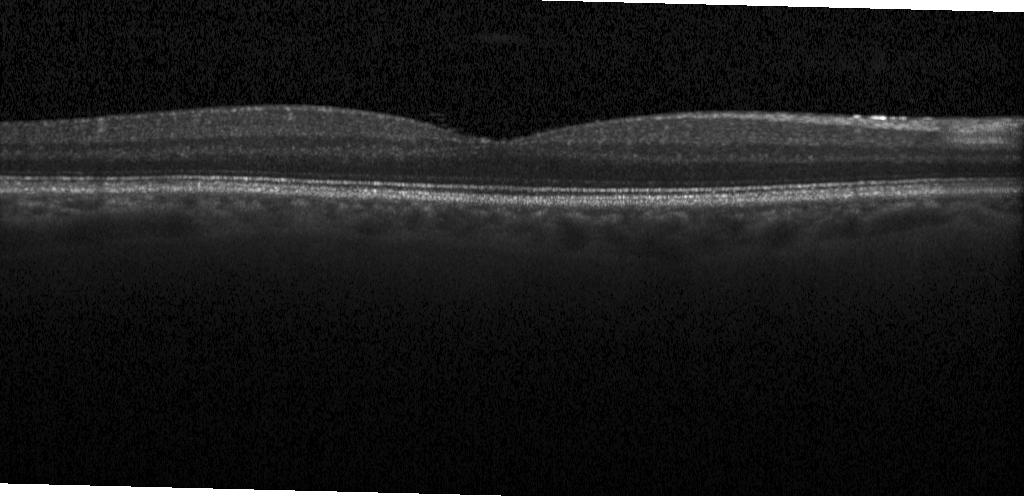 Retinal OCT B-scan.
Diagnosis: no choroidal neovascularization, diabetic macular edema, or drusen.